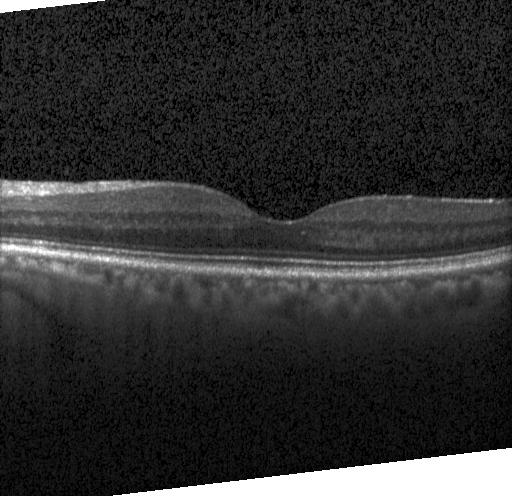 Heidelberg Spectralis; retinal OCT cross-section; through the macula — Finding: no evidence of choroidal neovascularization, diabetic macular edema, or drusen.